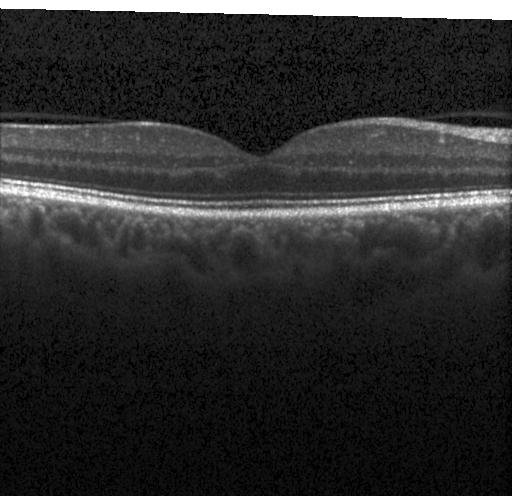

Impression: no choroidal neovascularization, no diabetic macular edema, and no drusen.